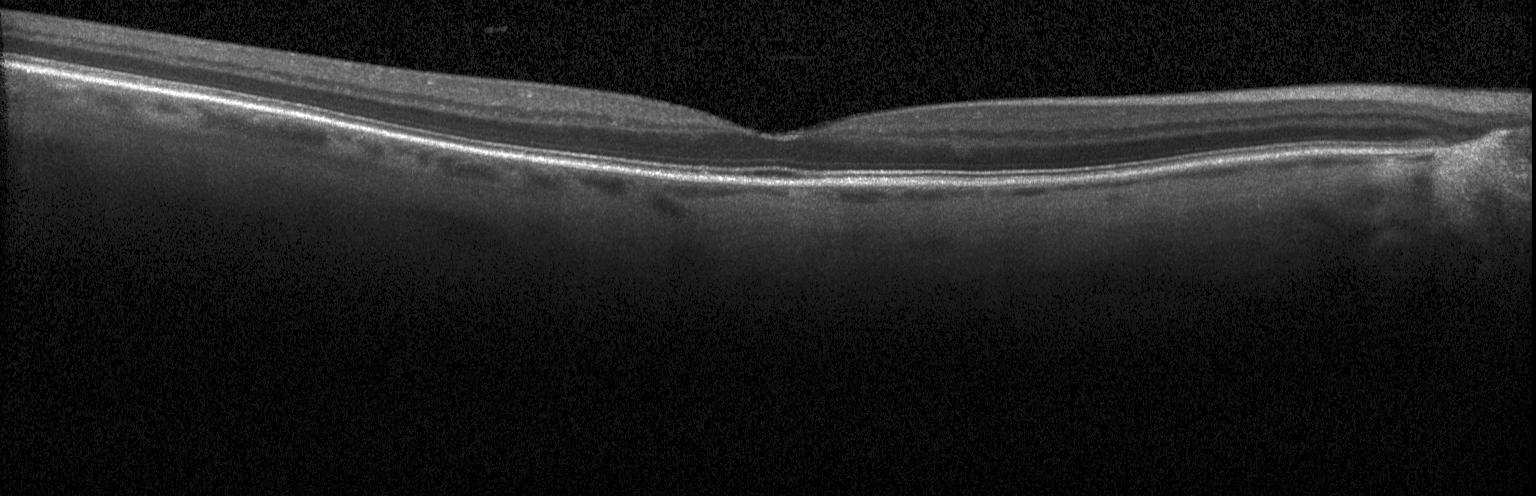
Dx: no choroidal neovascularization, diabetic macular edema, or drusen.